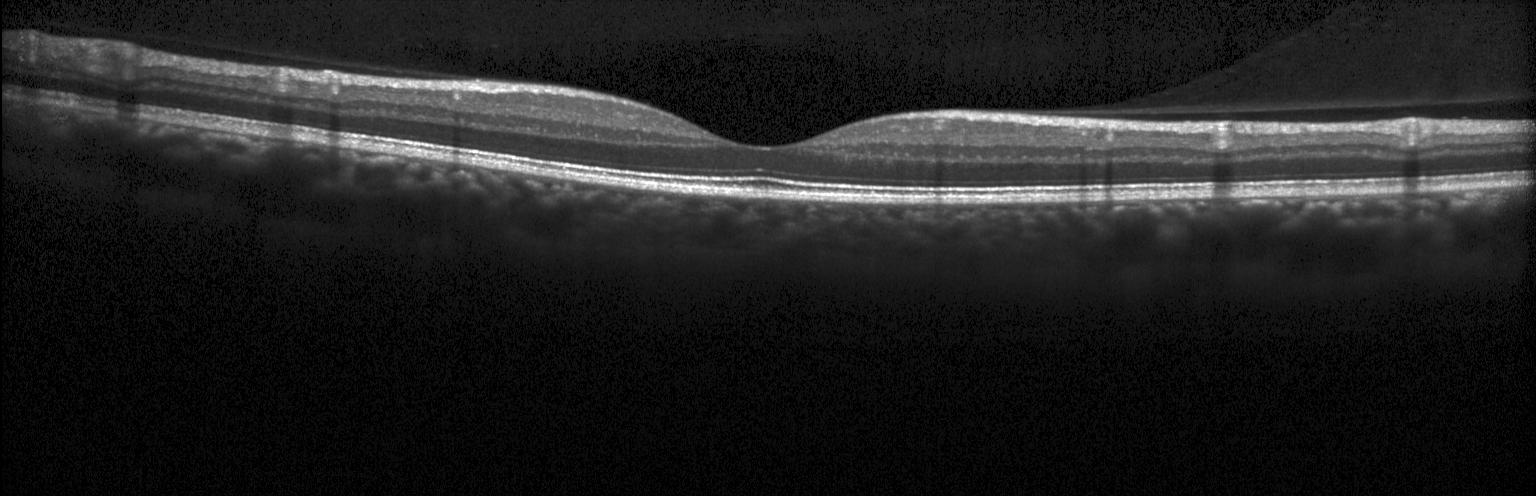 Acquired on a Heidelberg Spectralis. Spectral-domain optical coherence tomography. Retinal OCT B-scan — OCT finding: neither choroidal neovascularization, diabetic macular edema, nor drusen.